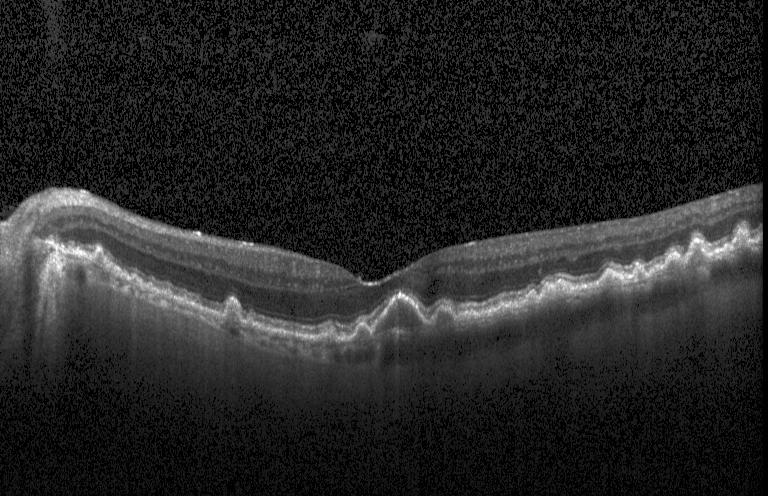 Through the macula · optical coherence tomography scan · Heidelberg Spectralis OCT system · spectral-domain optical coherence tomography.
OCT finding: multiple drusen.